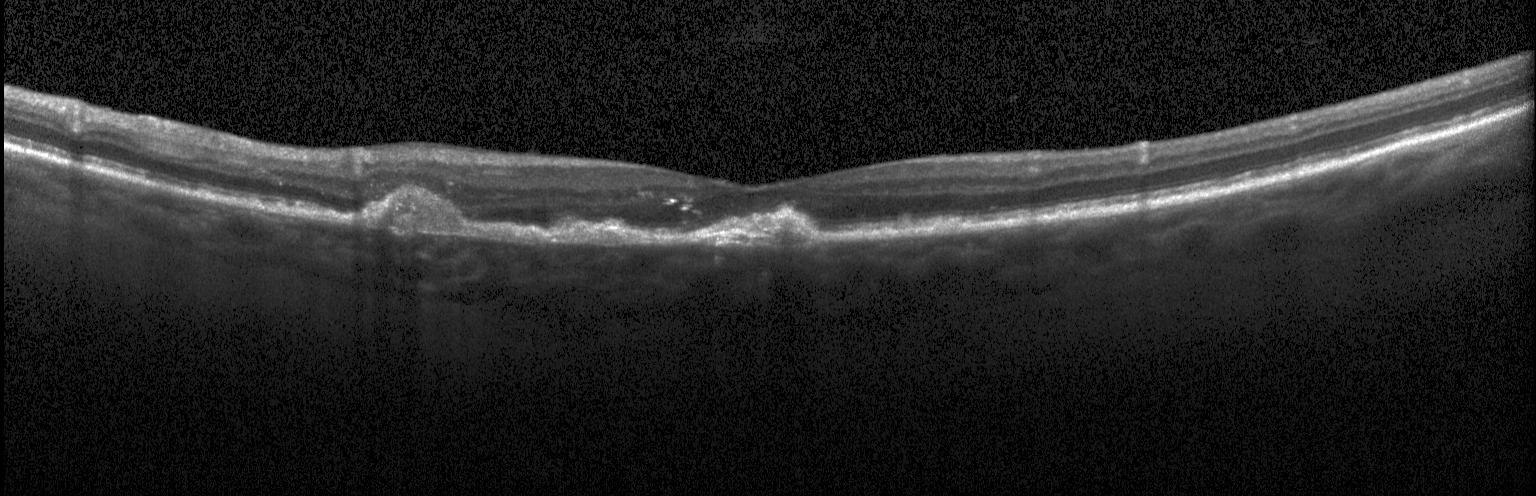 Macular OCT: a choroidal neovascular membrane.